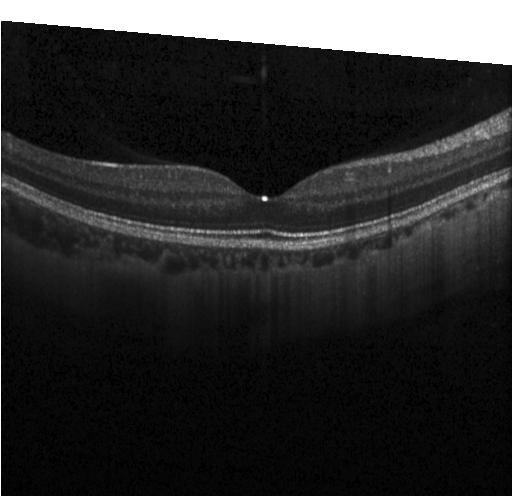
Fovea-centered · optical coherence tomography scan — This B-scan demonstrates no evidence of choroidal neovascularization, diabetic macular edema, or drusen.